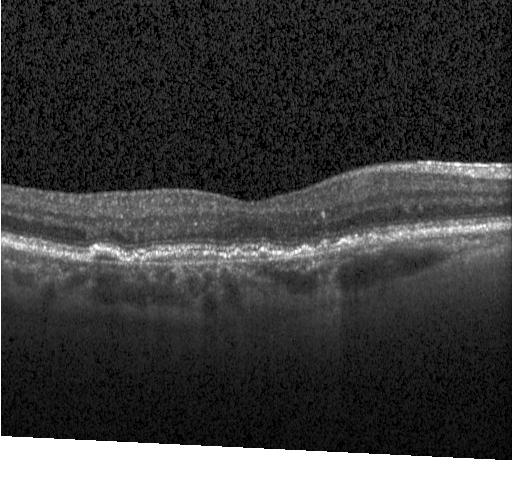
Through the macula; Heidelberg Spectralis OCT system; optical coherence tomography B-scan; spectral-domain OCT
The scan shows choroidal neovascularization (CNV).